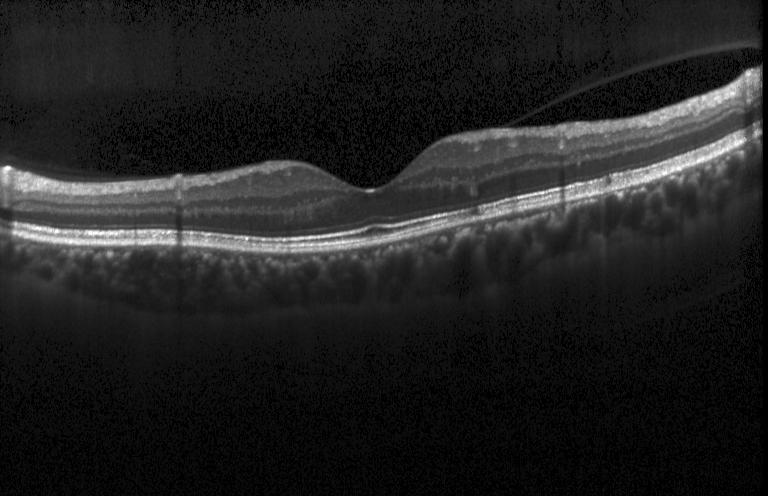
Finding: neither CNV, DME, nor drusen.